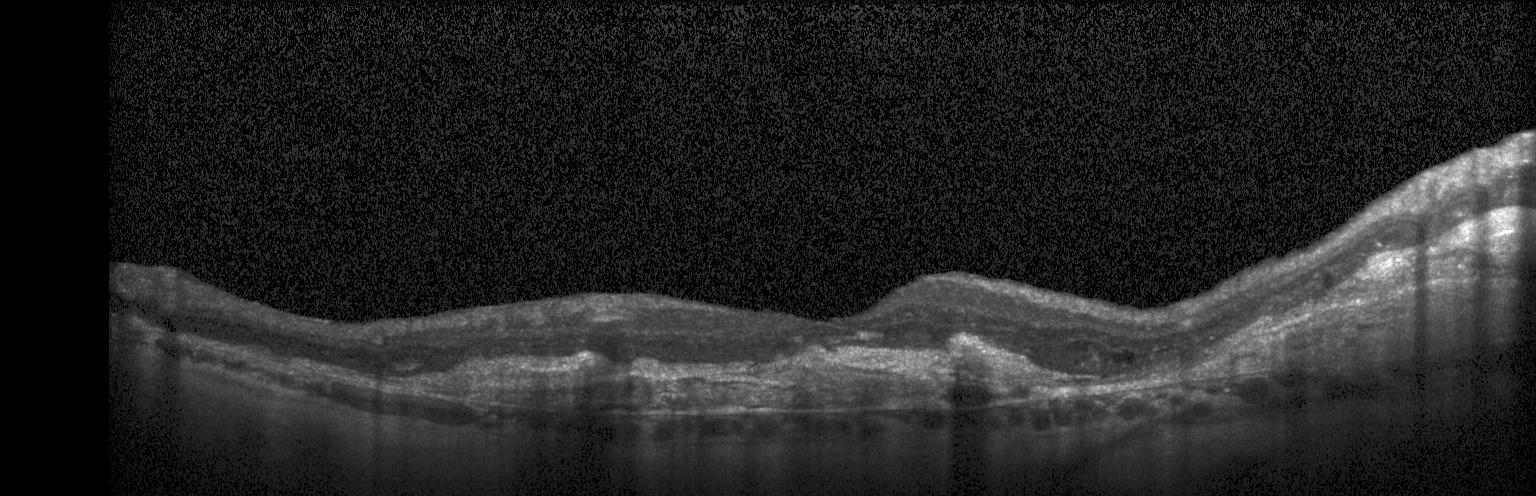 Assessment: a choroidal neovascular membrane.